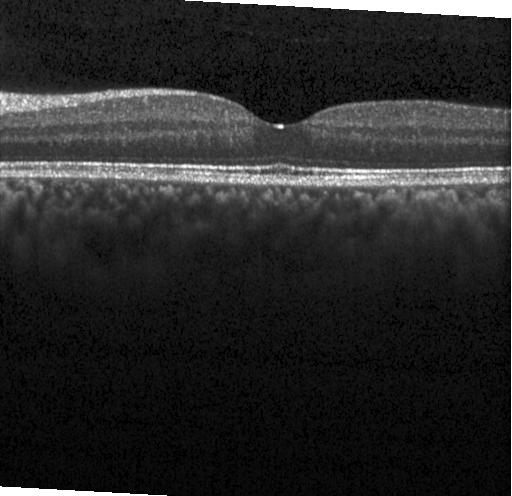

Spectral-domain OCT · optical coherence tomography scan
OCT finding: no choroidal neovascularization, diabetic macular edema, or drusen.